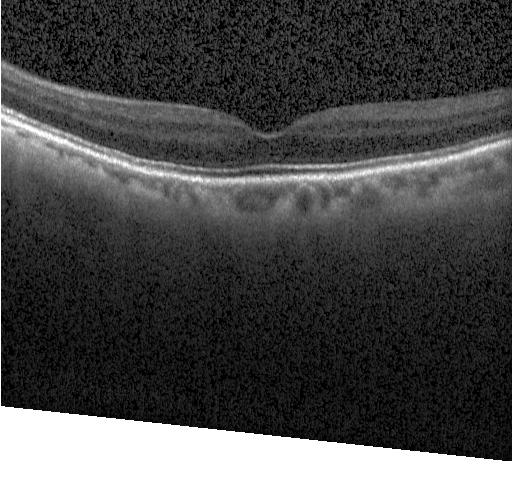

Retinal OCT cross-section. Instrument: Heidelberg Spectralis
Diagnosis: neither choroidal neovascularization, diabetic macular edema, nor drusen.